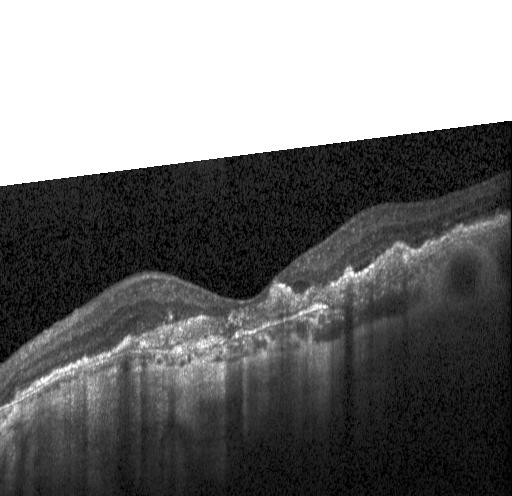

Diagnosis: a choroidal neovascular membrane.